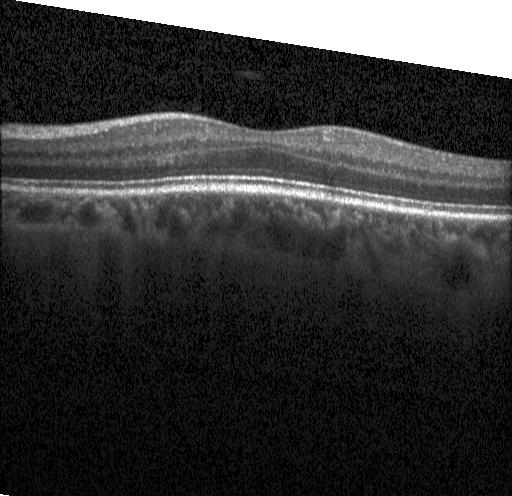 OCT B-scan showing no evidence of CNV, DME, or drusen.